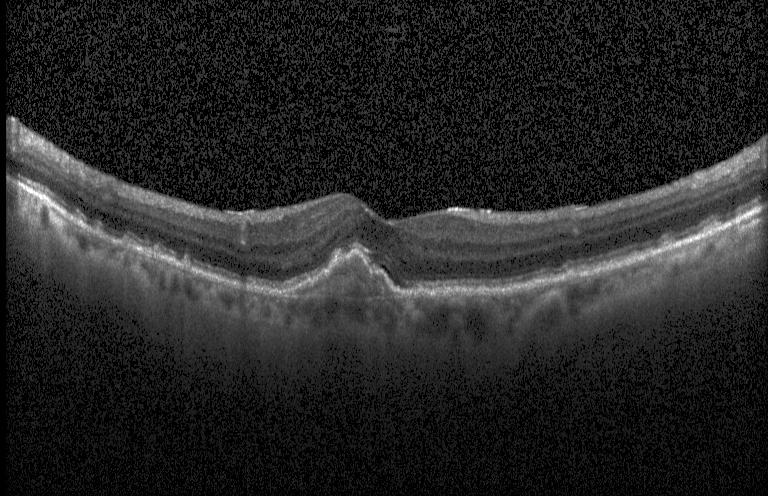
SD-OCT, retinal OCT cross-section. CNV.